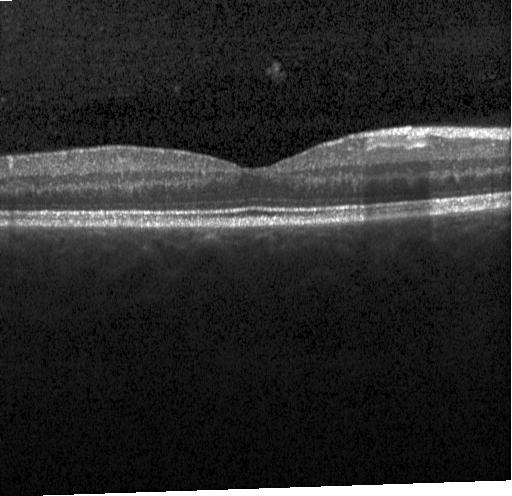
Macular OCT demonstrating no evidence of CNV, DME, or drusen.